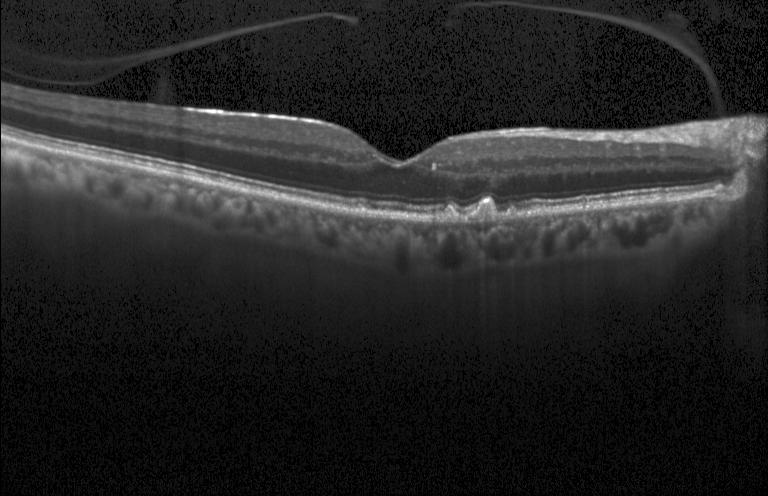
Assessment: sub-RPE drusenoid deposits.